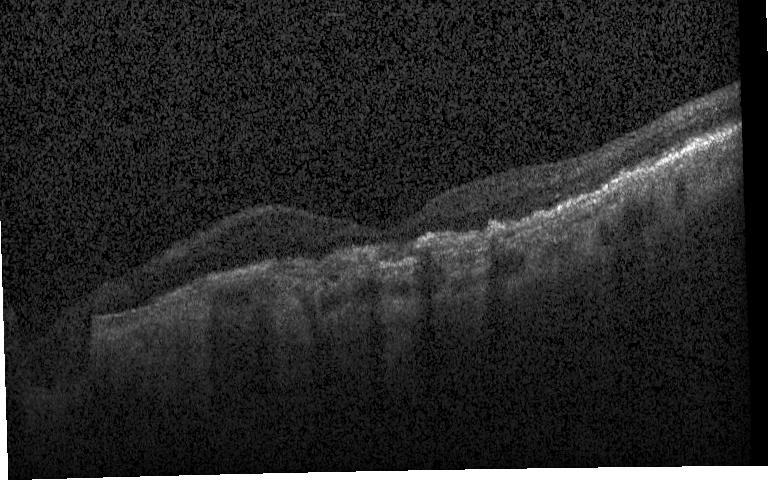

Dx: a choroidal neovascular membrane.